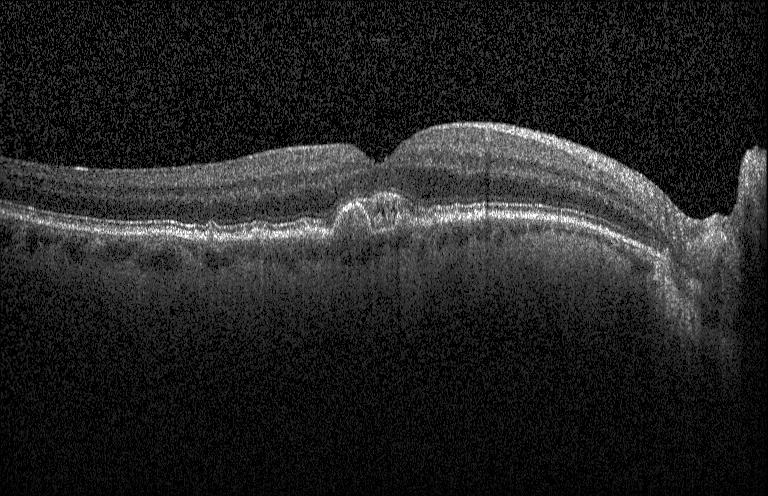

Spectral-domain OCT · centered on the fovea · optical coherence tomography B-scan
This B-scan demonstrates multiple drusen.